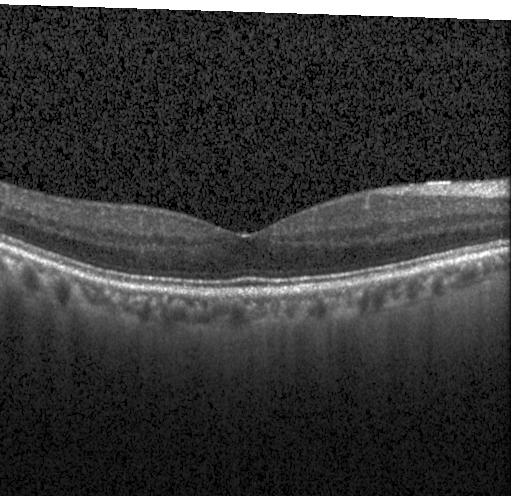
Spectral-domain OCT B-scan: no choroidal neovascularization, diabetic macular edema, or drusen.